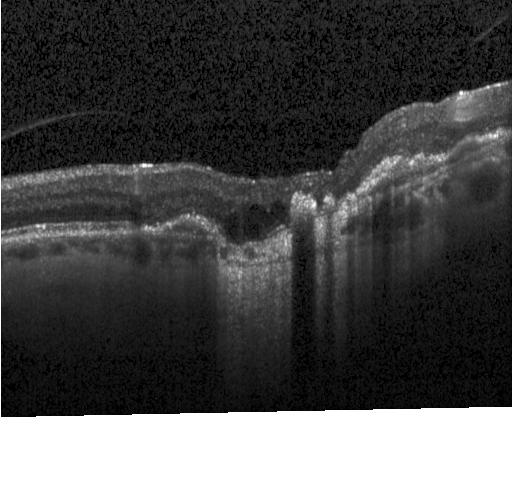 Diagnosis: a choroidal neovascular membrane.